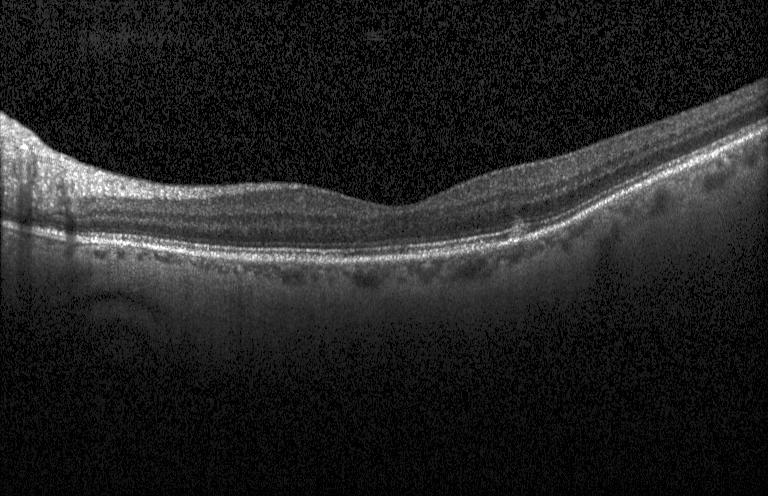
Instrument: Heidelberg Spectralis, retinal OCT cross-section — No choroidal neovascularization, no diabetic macular edema, and no drusen.